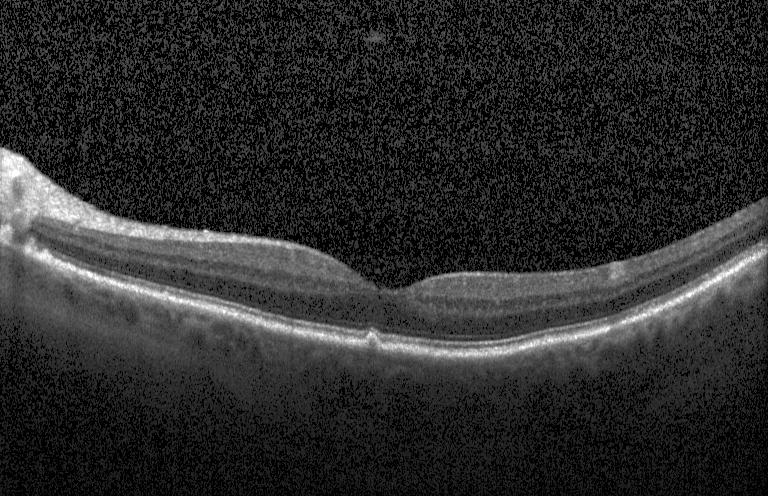 Optical coherence tomography scan; spectral-domain OCT; Heidelberg Spectralis. Dx: drusen.